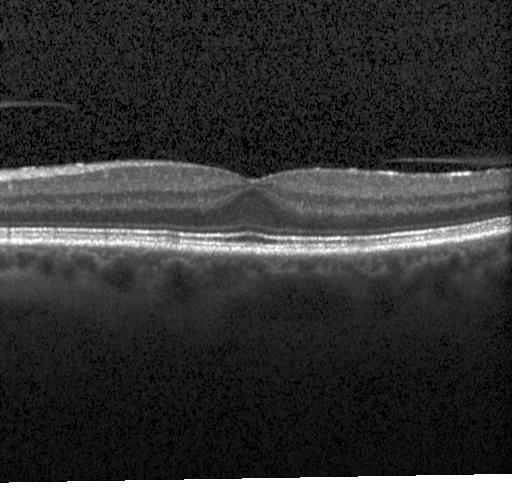

Impression: no choroidal neovascularization, no diabetic macular edema, and no drusen.